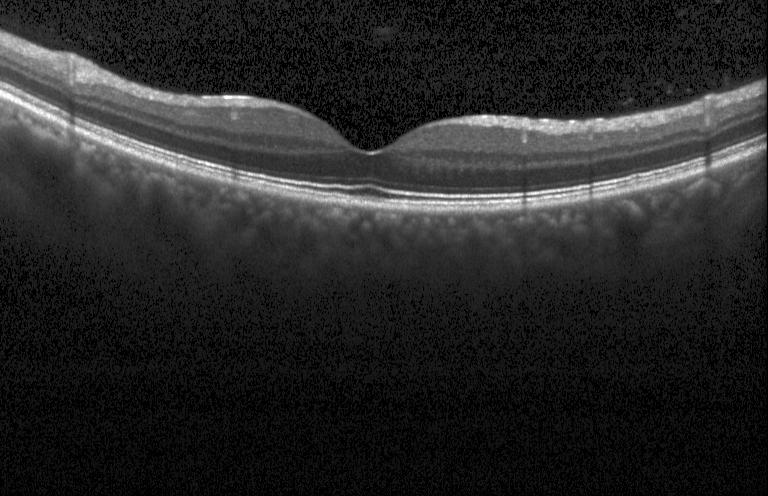

Spectral-domain OCT B-scan: neither CNV, DME, nor drusen.